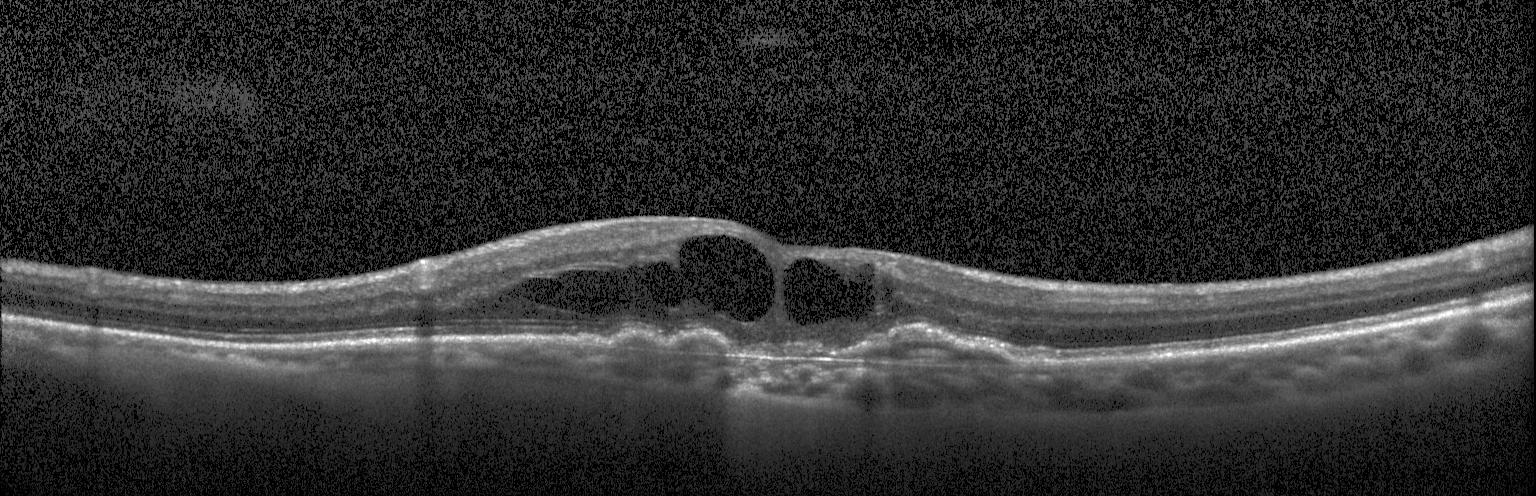

The scan shows CNV.